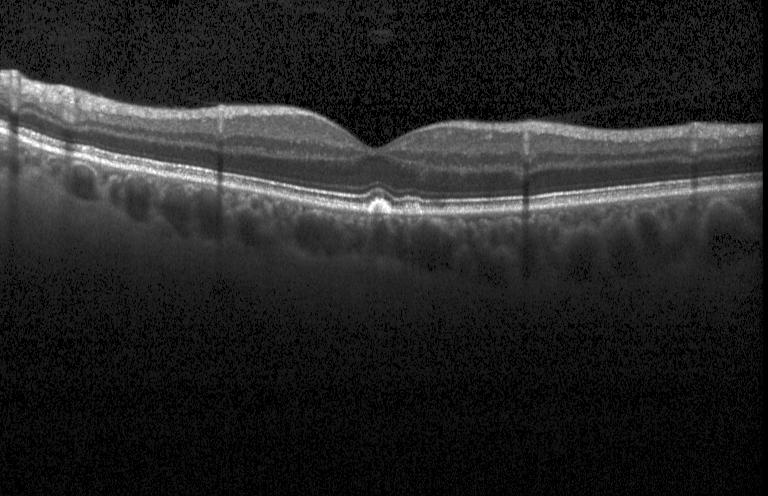
Through the macula. OCT B-scan
Finding: drusen.